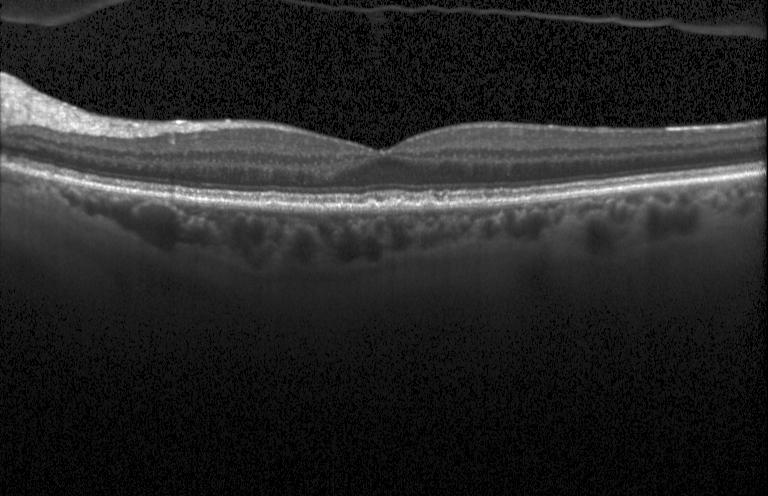

Macular OCT: drusen.